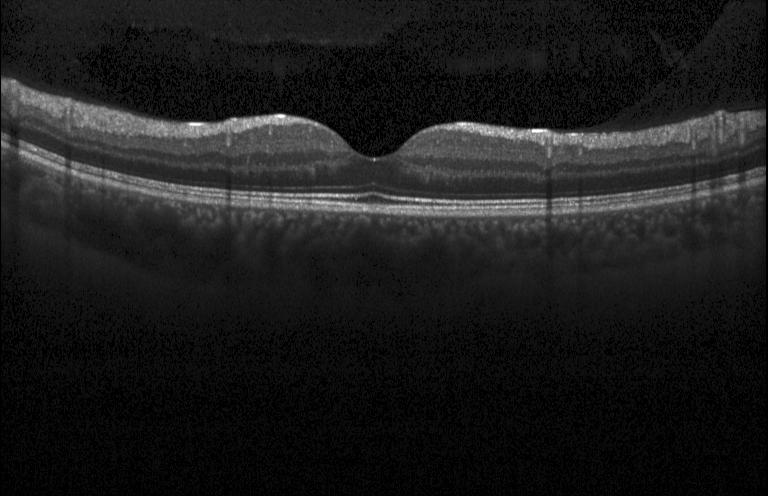

Diagnosis: no CNV, DME, or drusen.